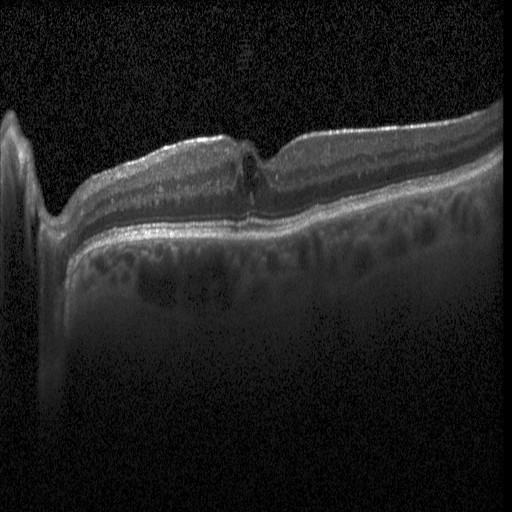
OCT line scan · instrument: Heidelberg Spectralis · SD-OCT · macular scan.
Assessment: diabetic macular edema.